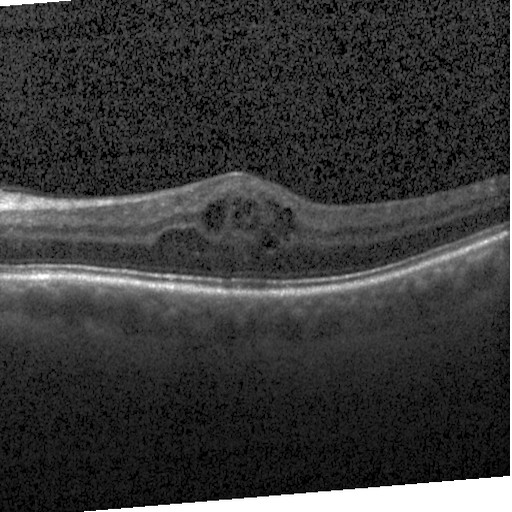 OCT line scan. Macular scan.
Diabetic macular edema (DME).